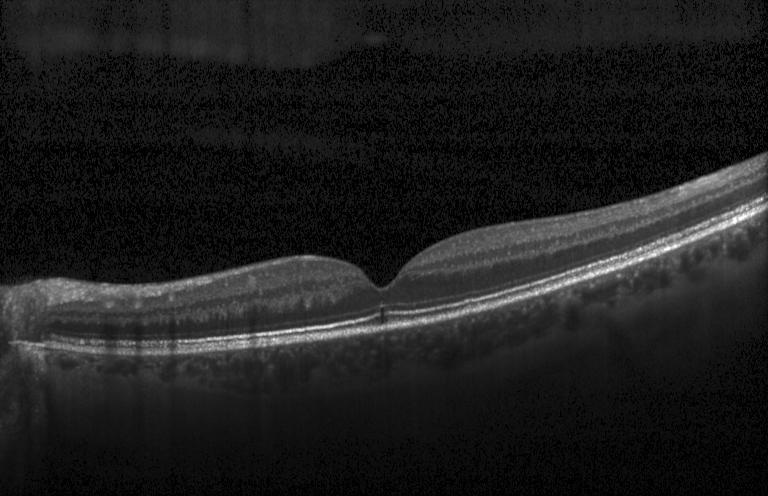 Spectral-domain optical coherence tomography · optical coherence tomography scan — Finding: neither choroidal neovascularization, diabetic macular edema, nor drusen.